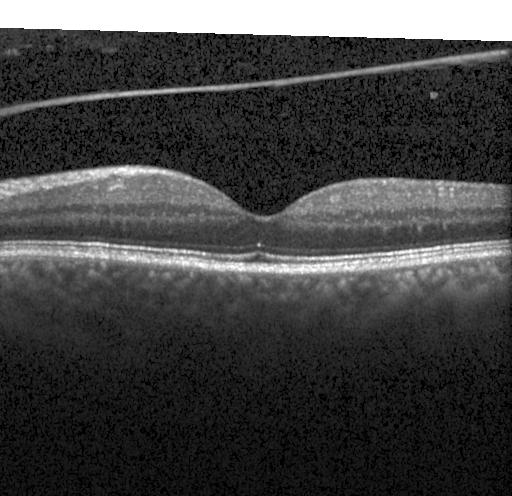
Retinal OCT cross-section. Spectral-domain OCT. Through the macula. Finding: neither CNV, DME, nor drusen.